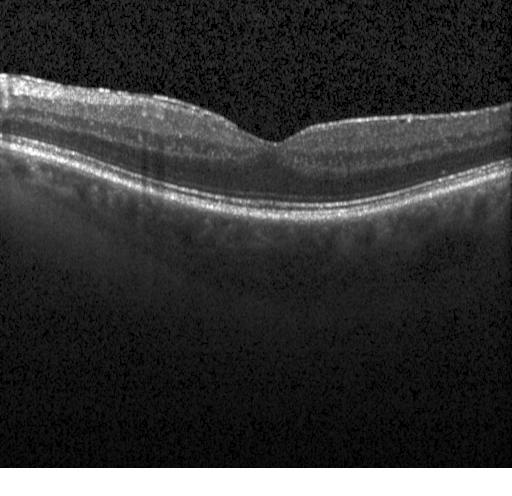
OCT line scan — Finding: no choroidal neovascularization, no diabetic macular edema, and no drusen.